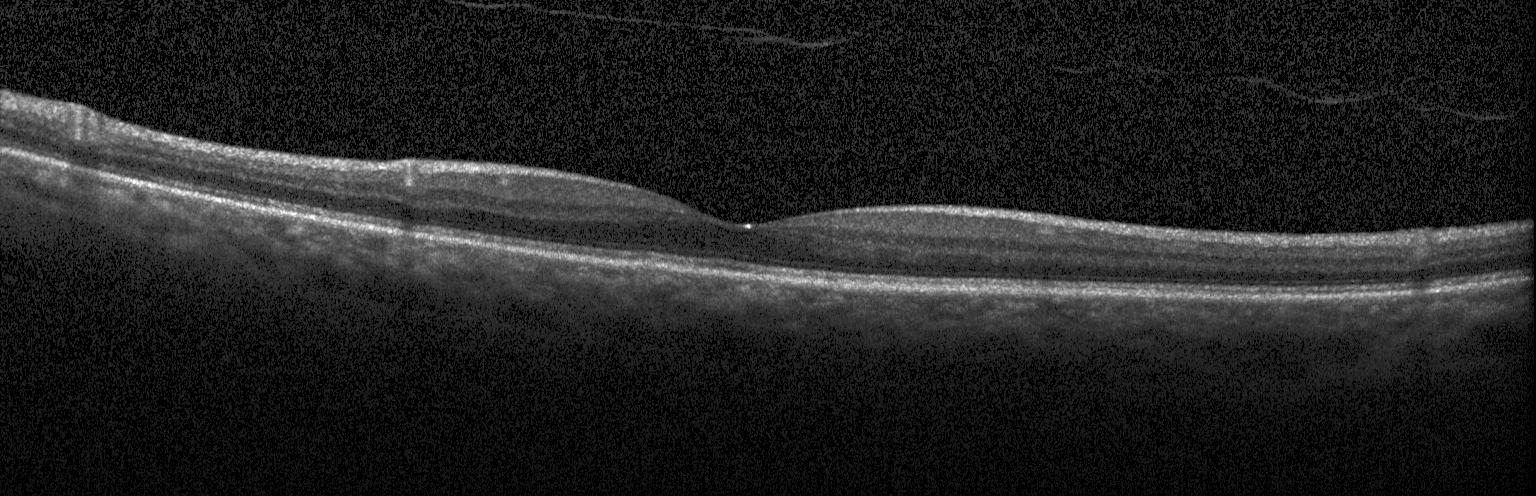 Retinal OCT B-scan. Horizontal scan through the fovea. Assessment: no choroidal neovascularization, diabetic macular edema, or drusen.